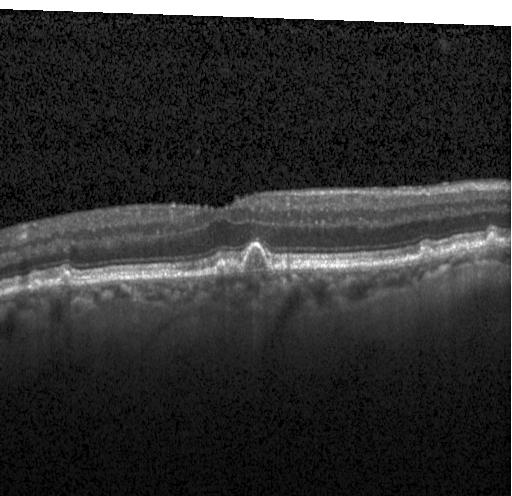 OCT scan showing multiple drusen.